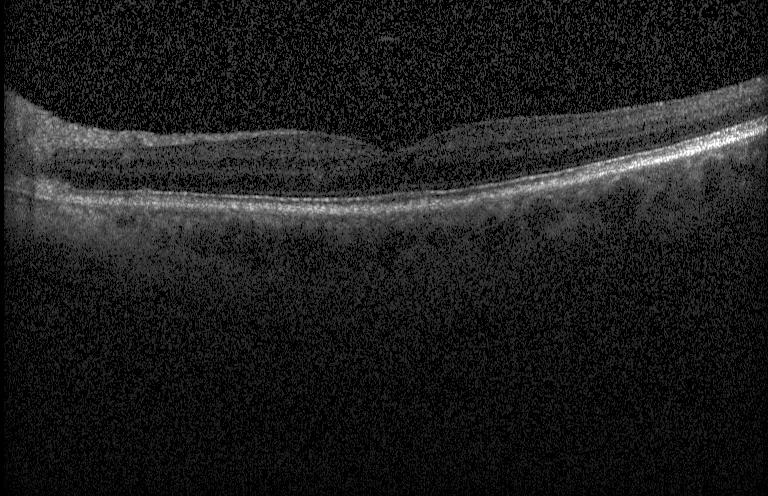
Impression: neither CNV, DME, nor drusen.